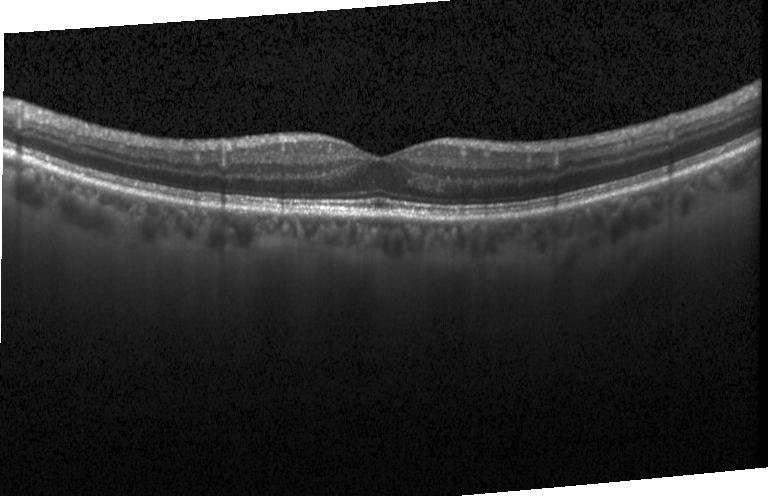

Finding: no choroidal neovascularization, diabetic macular edema, or drusen.